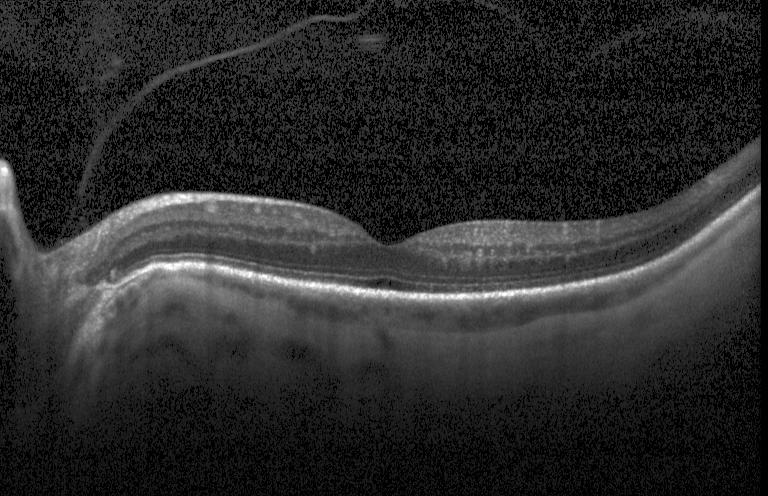 Optical coherence tomography scan — This B-scan demonstrates neither choroidal neovascularization, diabetic macular edema, nor drusen.